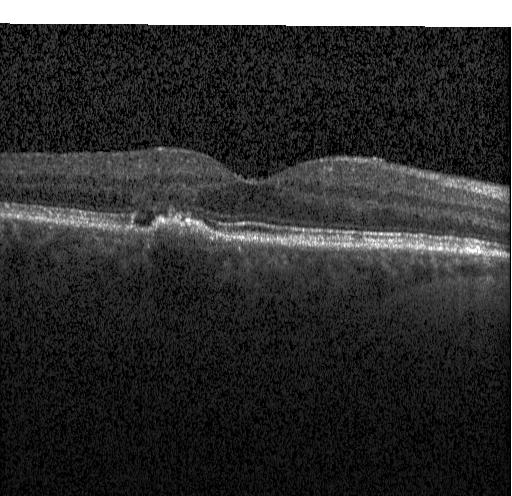
Instrument: Heidelberg Spectralis; spectral-domain optical coherence tomography; OCT B-scan — Finding: a choroidal neovascular membrane.